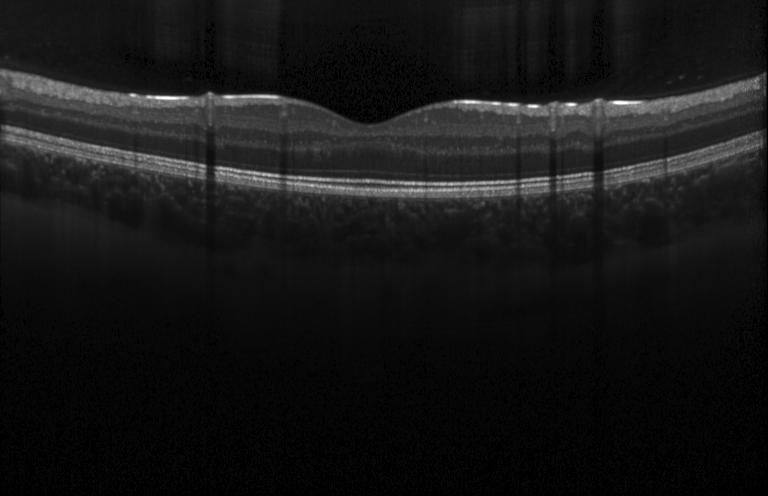
OCT B-scan — Impression: neither choroidal neovascularization, diabetic macular edema, nor drusen.